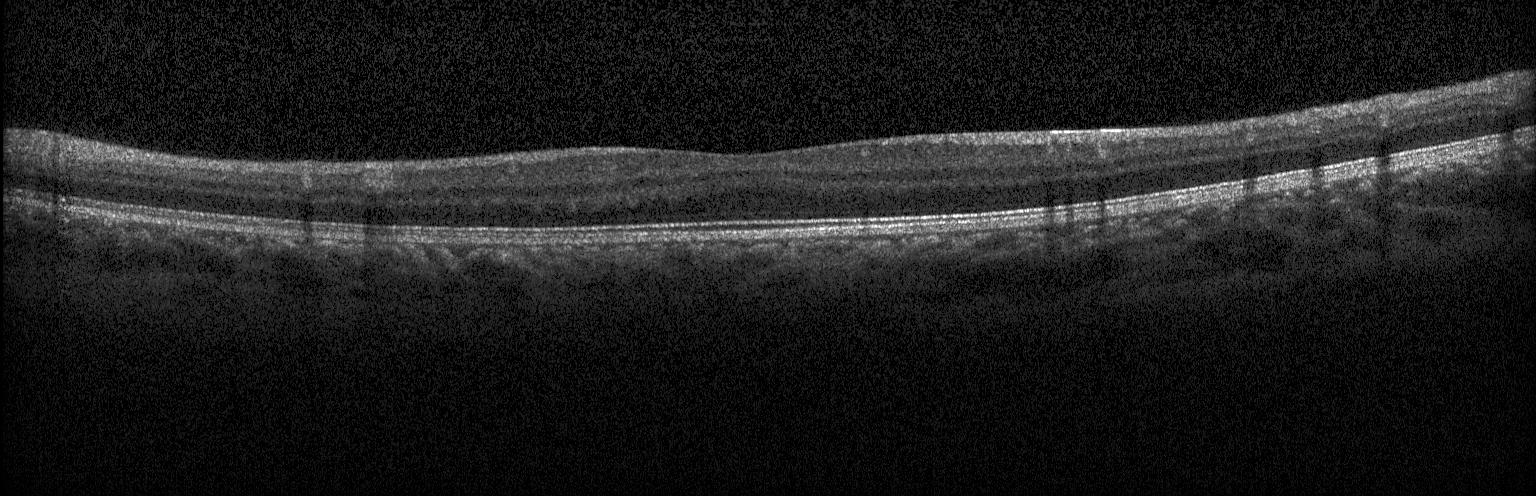 Heidelberg Spectralis OCT system; macular scan; spectral-domain optical coherence tomography; optical coherence tomography scan
Diagnosis: no evidence of choroidal neovascularization, diabetic macular edema, or drusen.